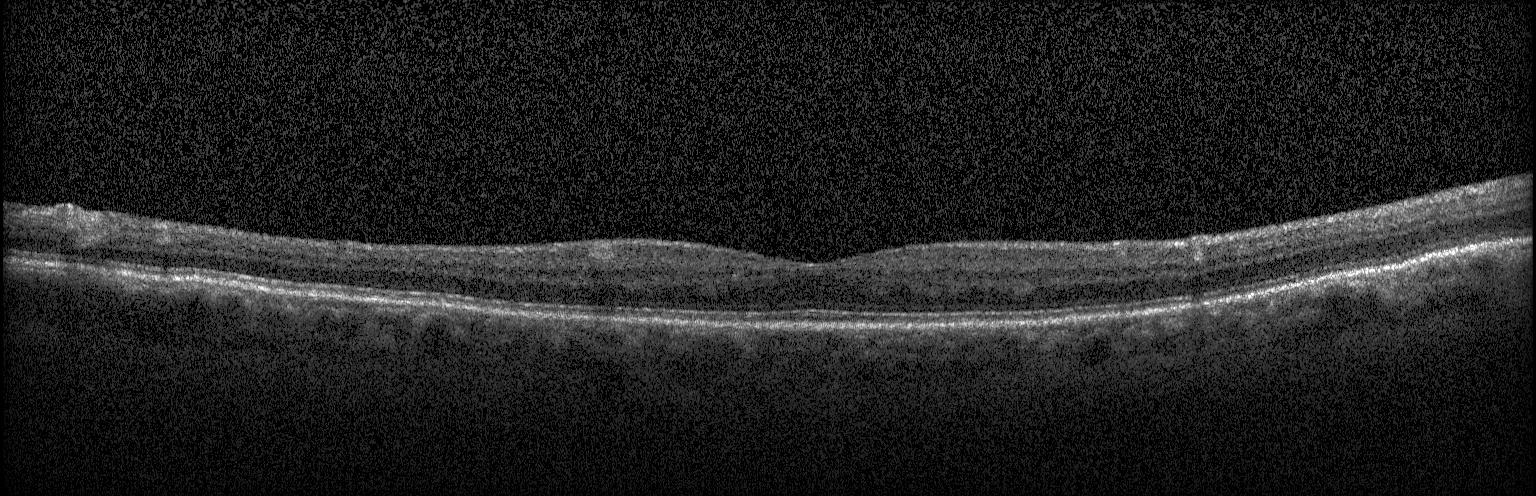 Optical coherence tomography B-scan, SD-OCT, acquired on a Heidelberg Spectralis, macular scan.
Dx: no choroidal neovascularization, no diabetic macular edema, and no drusen.